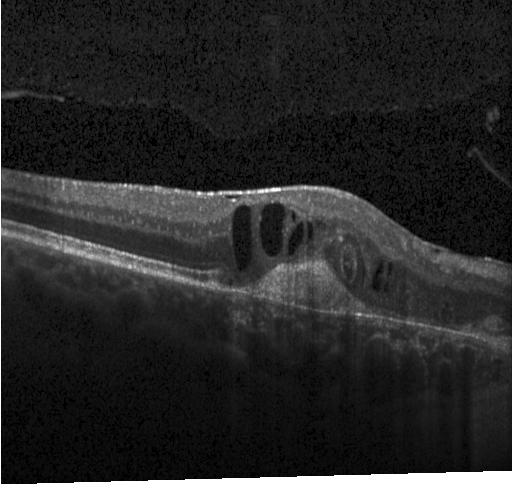

Finding: choroidal neovascularization.